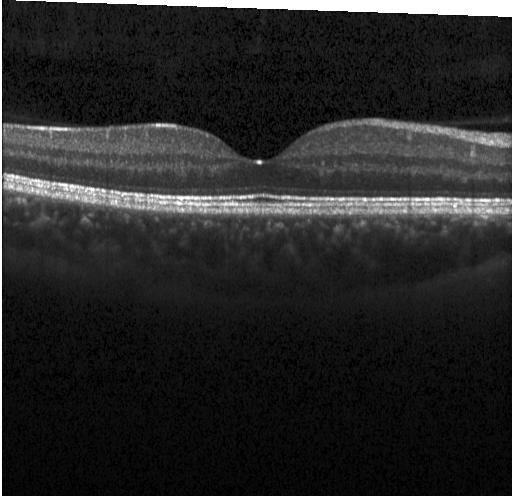

Heidelberg Spectralis OCT system · retinal OCT cross-section · spectral-domain optical coherence tomography — Diagnosis: no CNV, no DME, and no drusen.